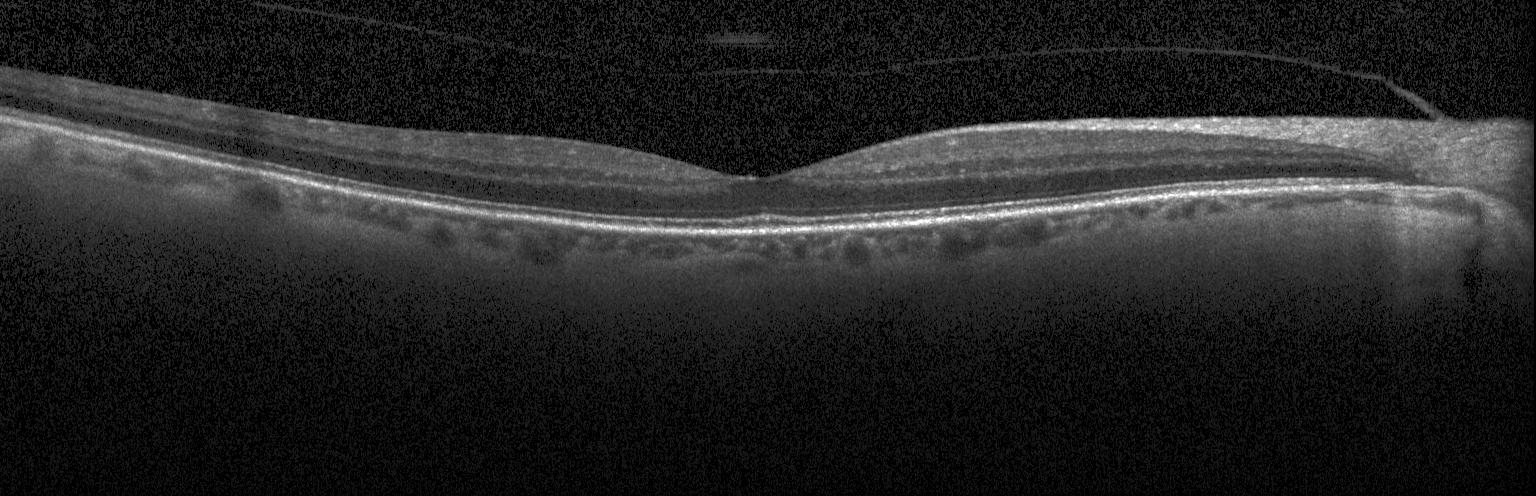 Optical coherence tomography scan. Acquired on a Heidelberg Spectralis. Horizontal scan through the fovea — Finding: no CNV, DME, or drusen.